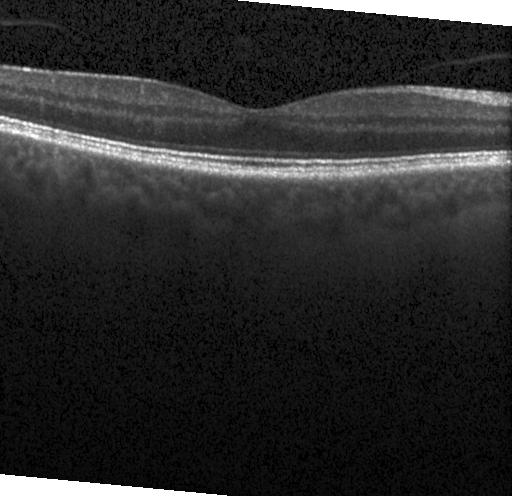
Retinal OCT B-scan · horizontal scan through the fovea · SD-OCT · acquired on a Heidelberg Spectralis.
This B-scan demonstrates no evidence of choroidal neovascularization, diabetic macular edema, or drusen.